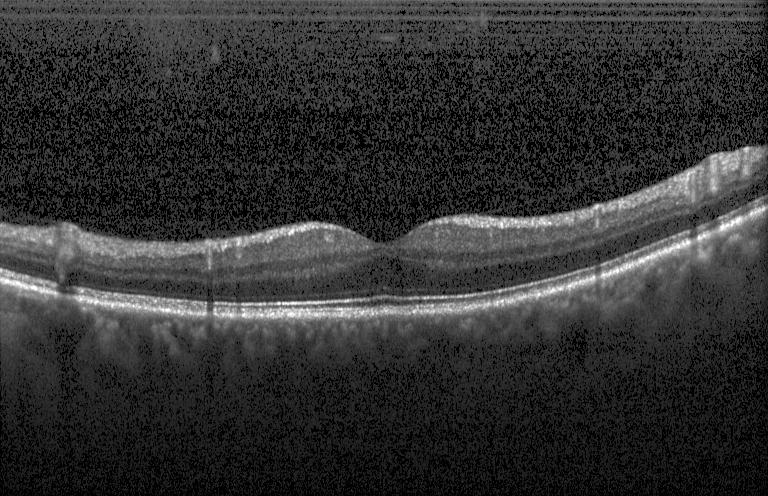

Optical coherence tomography scan.
Diagnosis: neither CNV, DME, nor drusen.